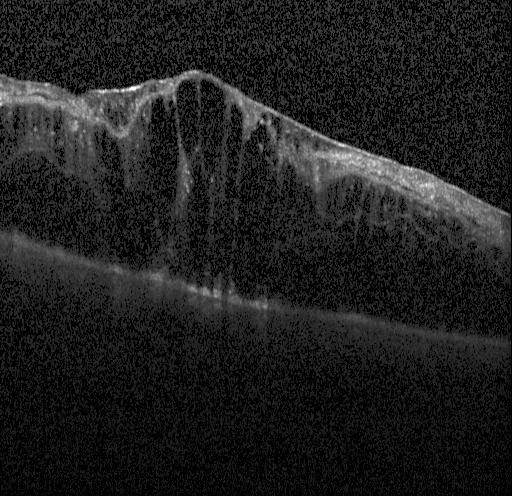

Acquired on a Heidelberg Spectralis, macular scan, spectral-domain optical coherence tomography, OCT B-scan
Finding: diabetic macular edema.